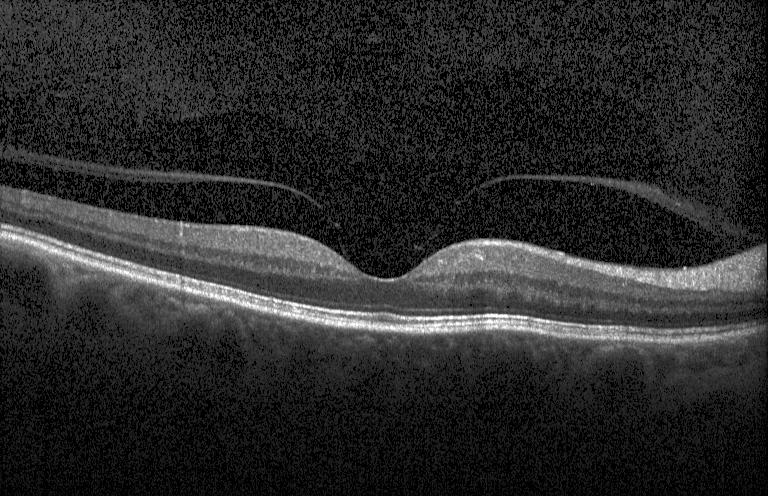 Impression: no choroidal neovascularization, diabetic macular edema, or drusen.